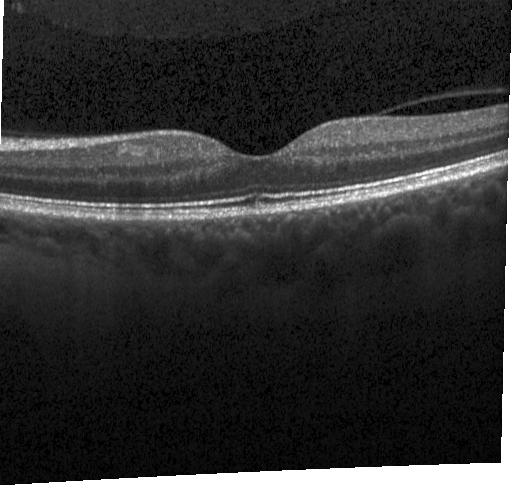 OCT B-scan; Heidelberg Spectralis OCT system. Macular OCT: neither CNV, DME, nor drusen.